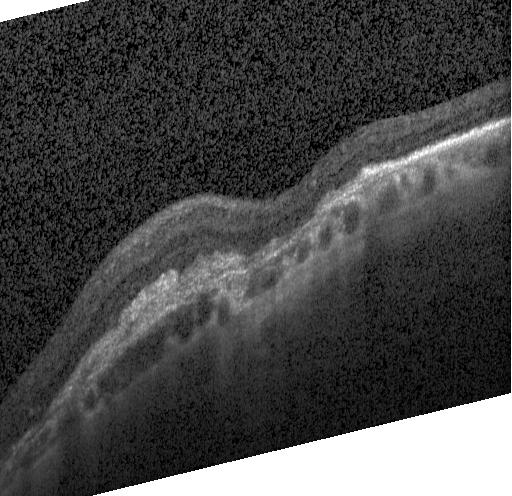

Diagnosis: choroidal neovascularization (CNV).